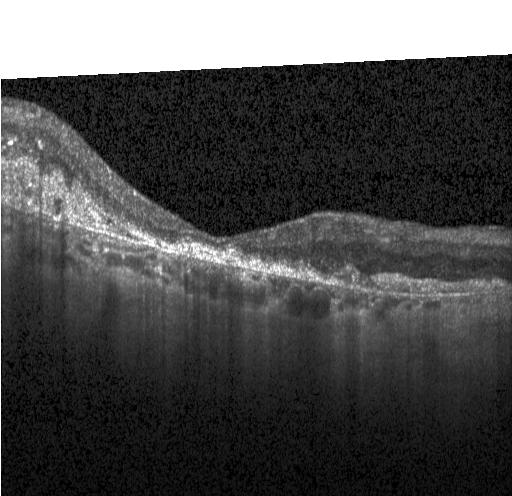

Macular OCT: a choroidal neovascular membrane.